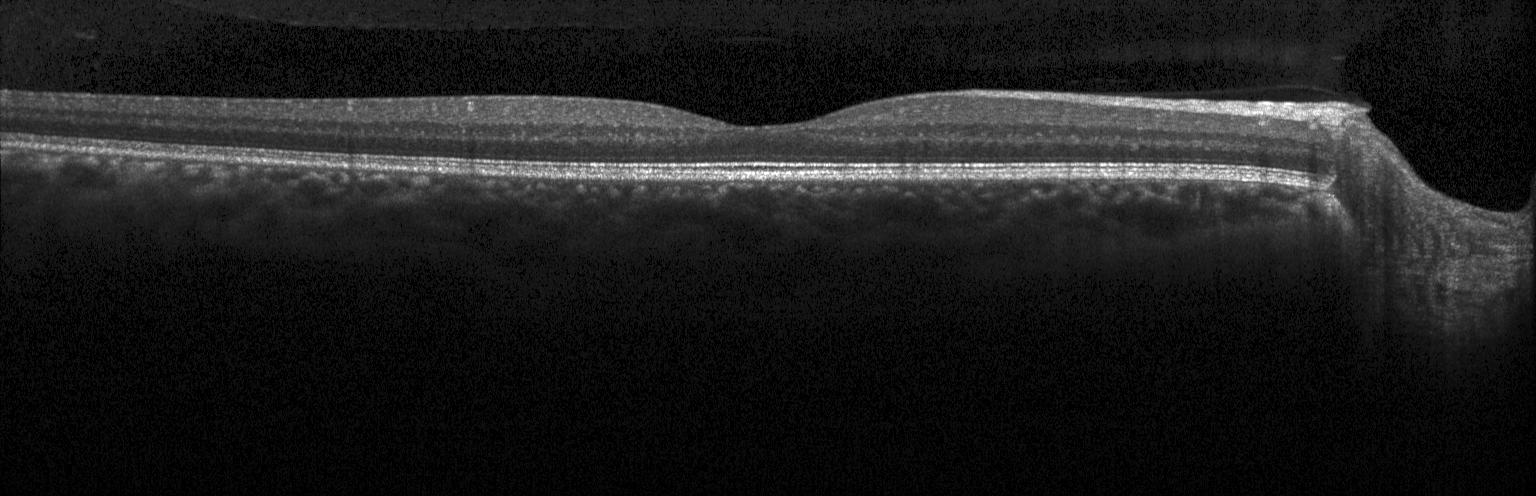

Finding: neither choroidal neovascularization, diabetic macular edema, nor drusen.